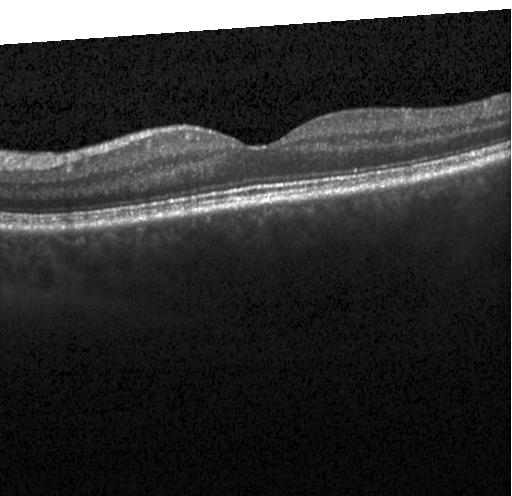 Through the macula; acquired on a Heidelberg Spectralis; optical coherence tomography B-scan. Diagnosis: no CNV, no DME, and no drusen.